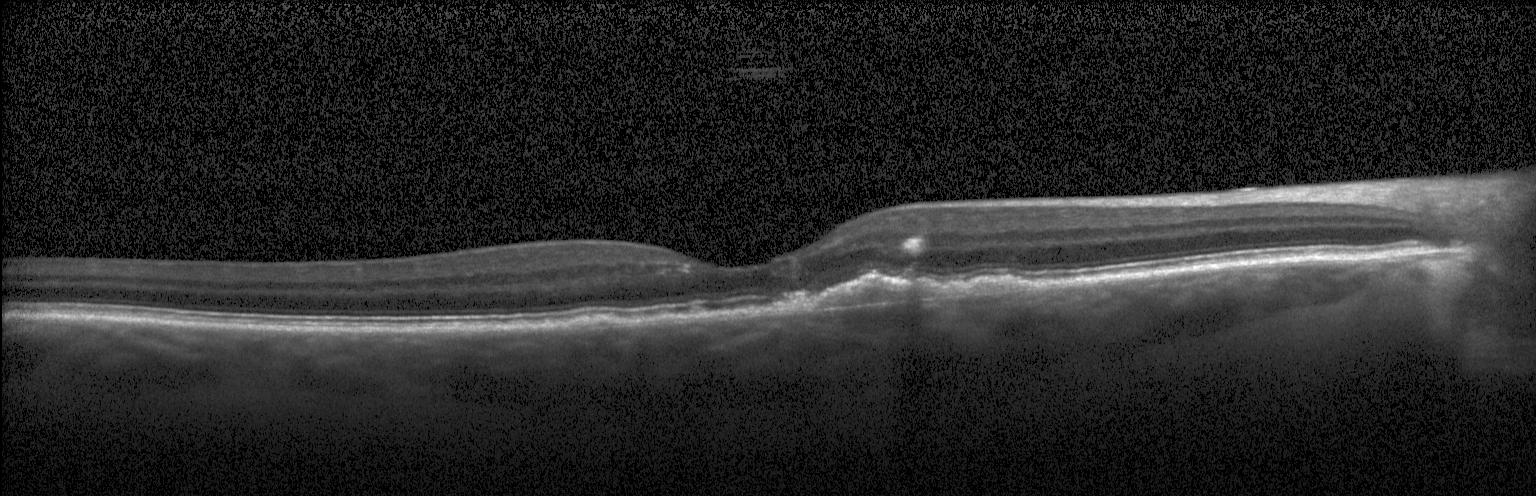 This B-scan demonstrates CNV.